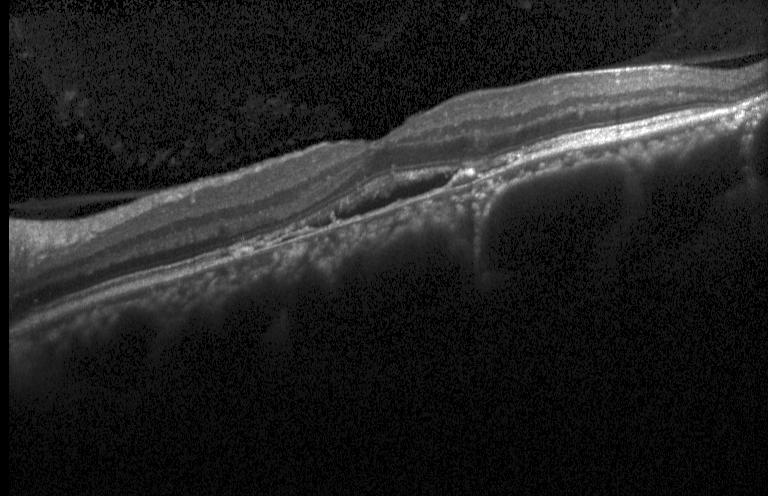

Impression: choroidal neovascularization (CNV).